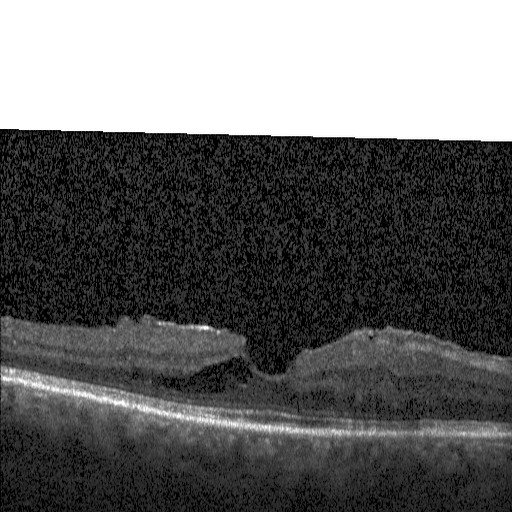
Retinal OCT cross-section showing DME.